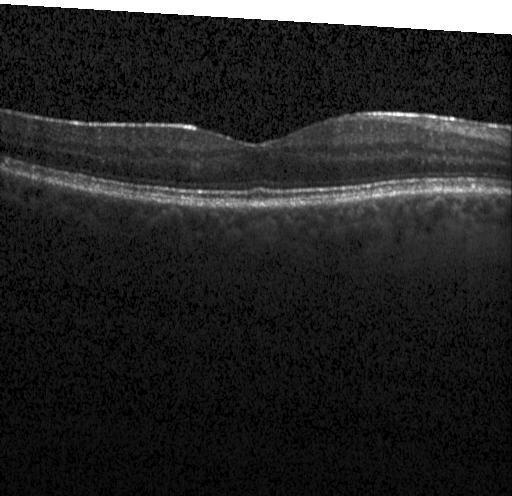

This B-scan demonstrates neither choroidal neovascularization, diabetic macular edema, nor drusen.